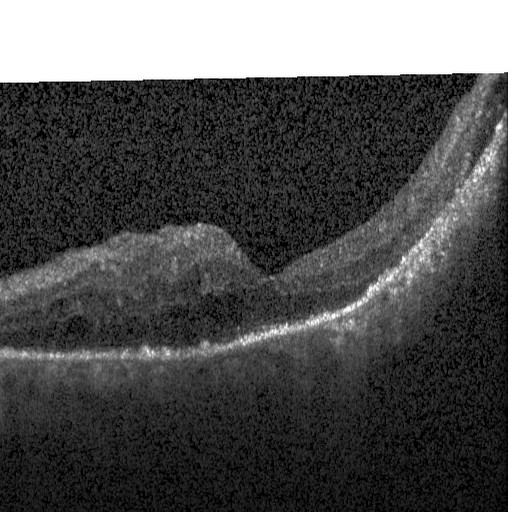

Finding: diabetic macular edema.